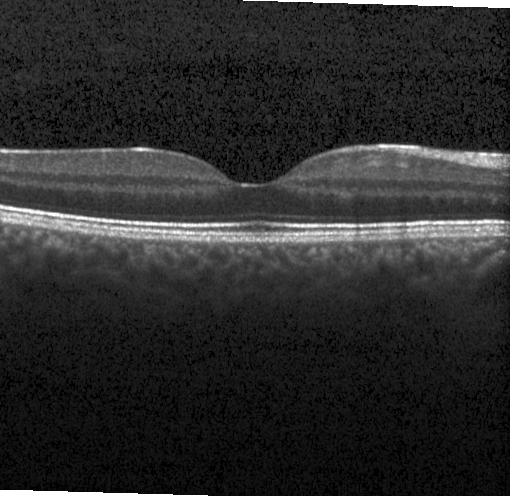 Diagnosis: no evidence of choroidal neovascularization, diabetic macular edema, or drusen.